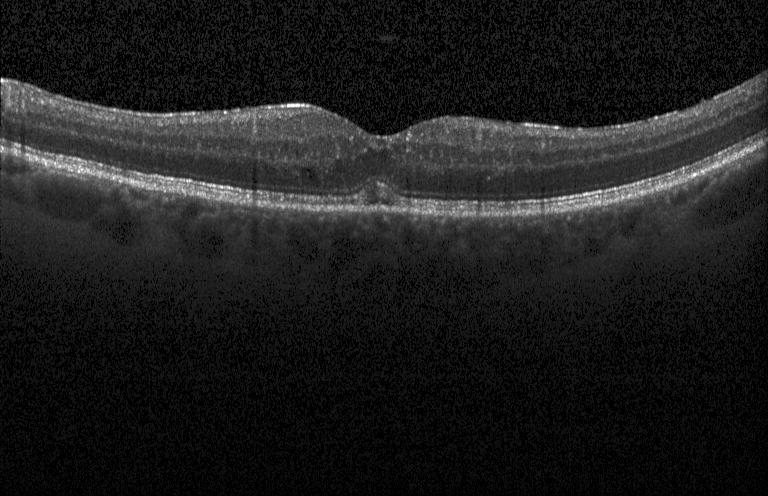
Heidelberg Spectralis OCT system; retinal OCT cross-section; macular scan.
The scan shows DME.